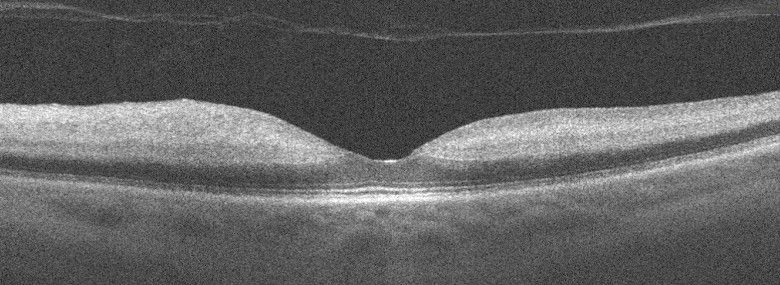 Retinal OCT cross-section · Optovue Avanti RTVue XR
Impression: retinal artery occlusion (RAO).